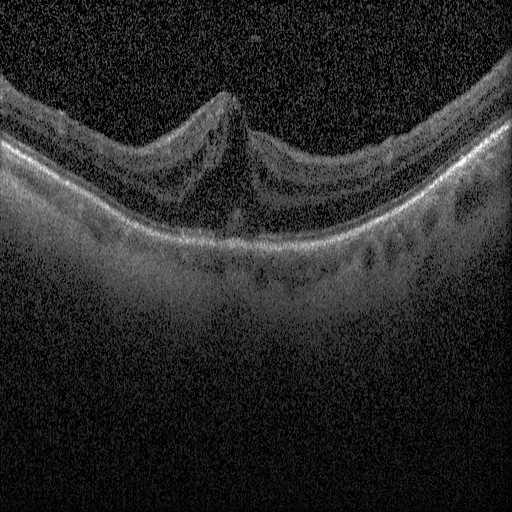

The scan shows diabetic macular edema.